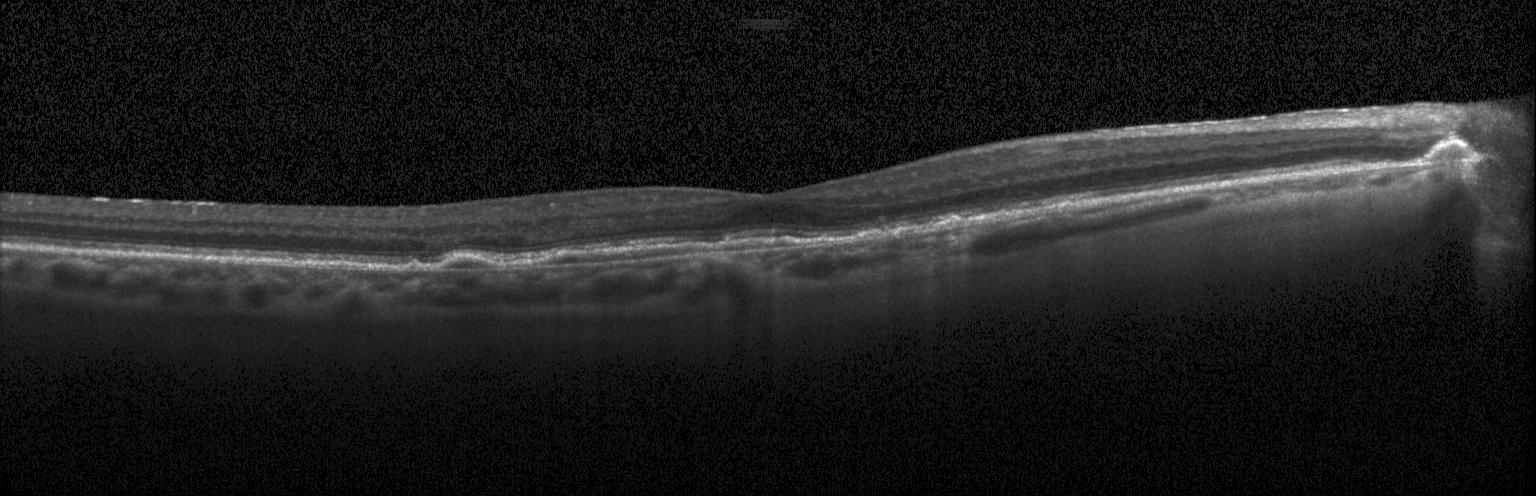
Assessment: choroidal neovascularization.